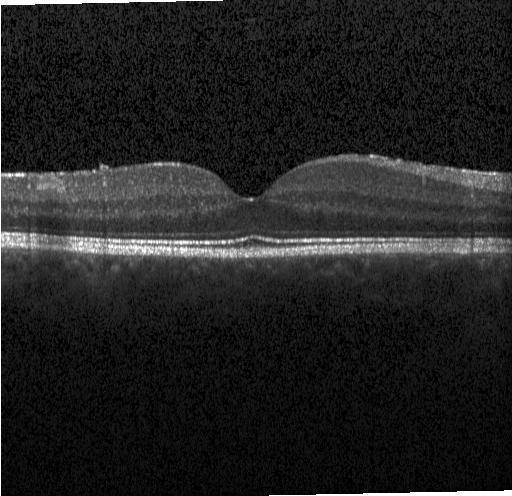 Macular scan, retinal OCT B-scan, spectral-domain OCT, acquired on a Heidelberg Spectralis
Diagnosis: neither choroidal neovascularization, diabetic macular edema, nor drusen.